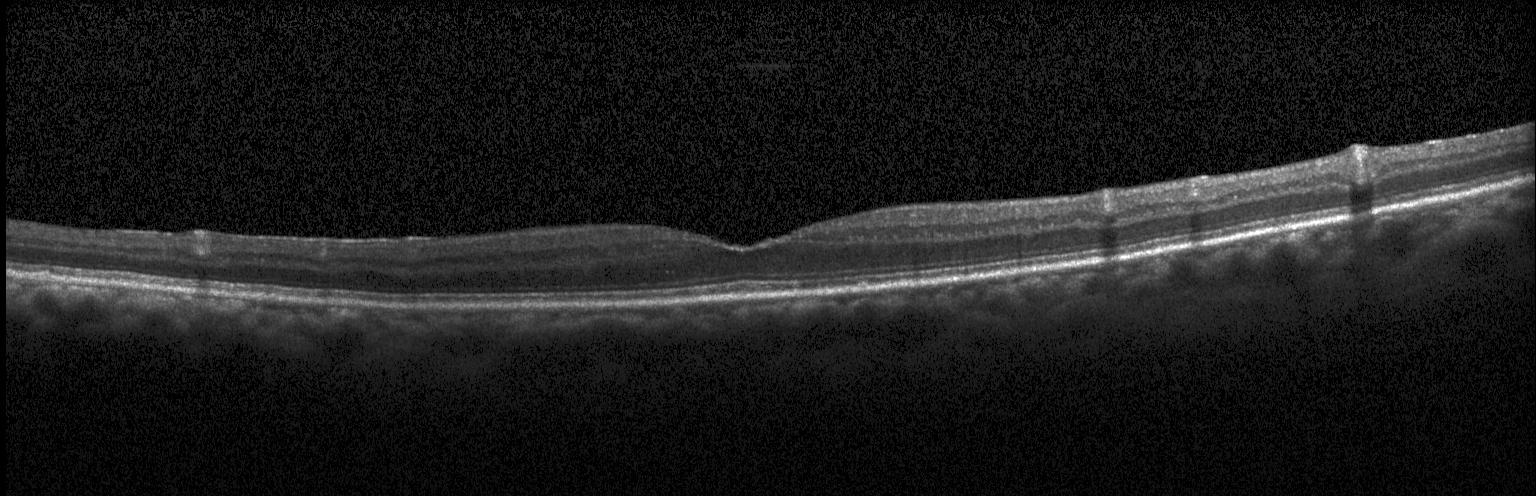
Spectral-domain OCT B-scan: neither CNV, DME, nor drusen.